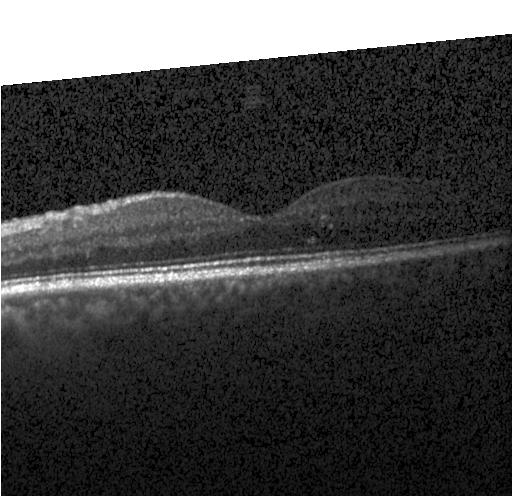

OCT line scan — Impression: no choroidal neovascularization, diabetic macular edema, or drusen.